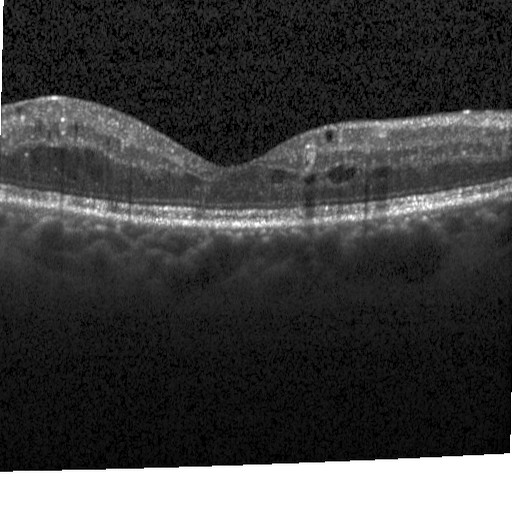

Retinal OCT cross-section showing diabetic macular edema.